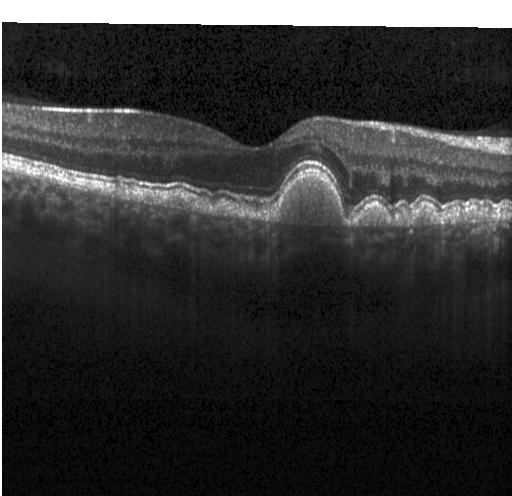

Optical coherence tomography scan
This B-scan demonstrates drusen.